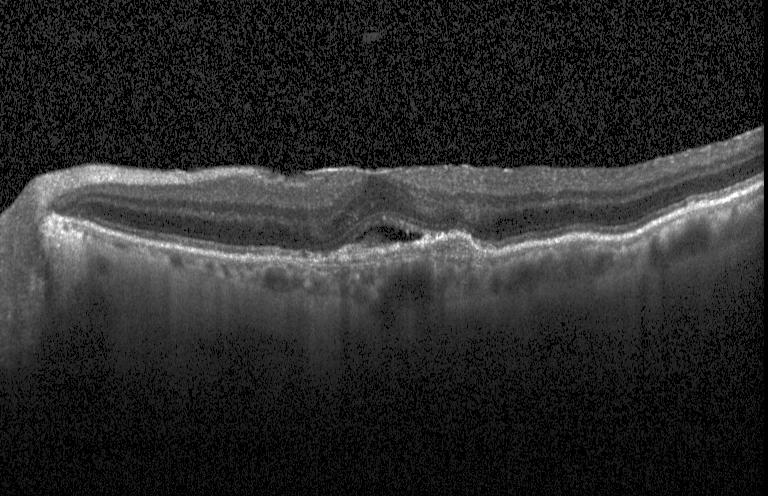 Finding: CNV.